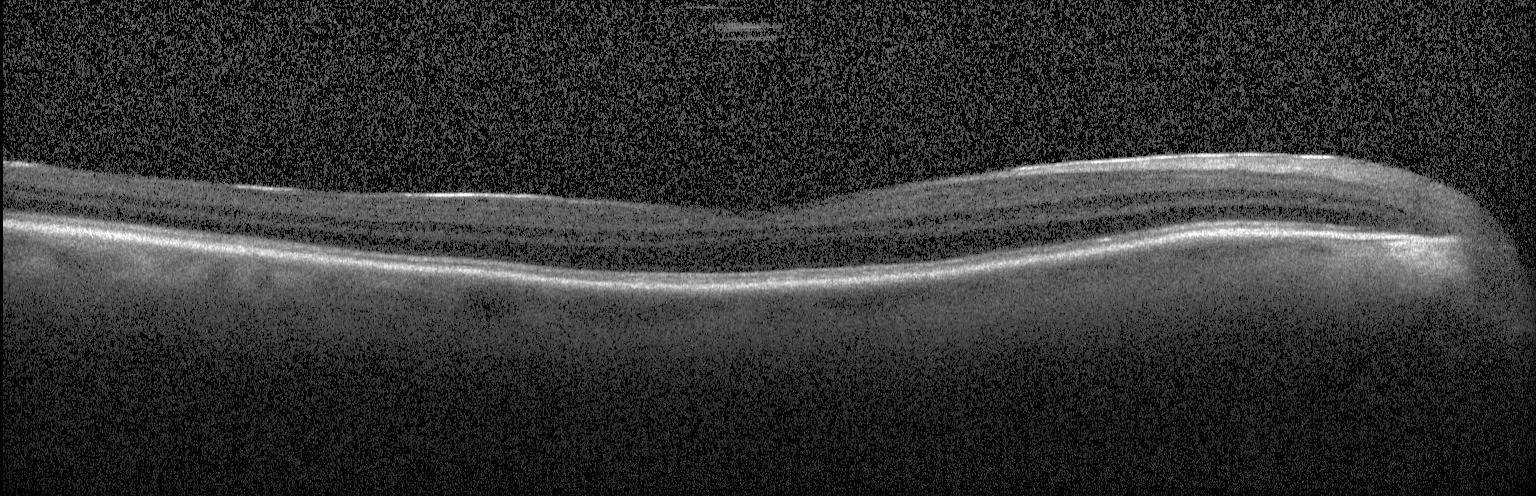
Spectral-domain OCT B-scan: no CNV, DME, or drusen.